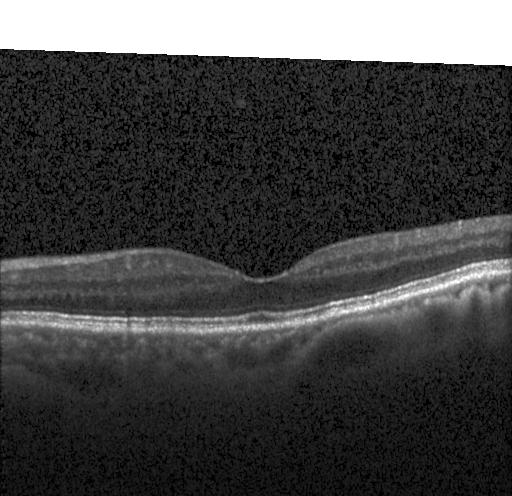 Optical coherence tomography B-scan
This B-scan demonstrates no choroidal neovascularization, no diabetic macular edema, and no drusen.